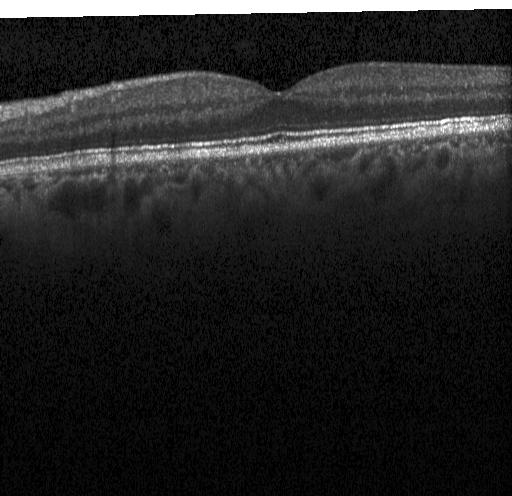

Impression: no choroidal neovascularization, diabetic macular edema, or drusen.